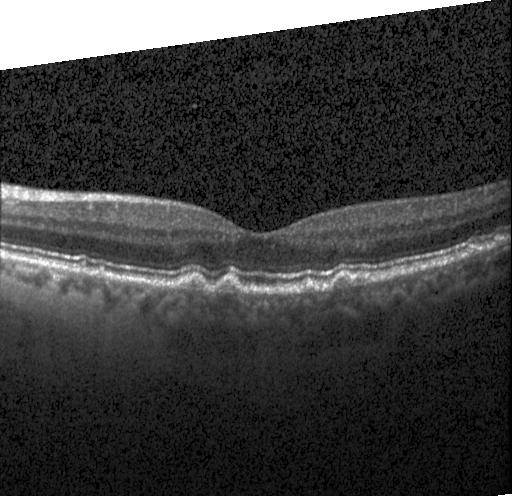 Optical coherence tomography B-scan · spectral-domain OCT · macular scan · acquired on a Heidelberg Spectralis
The scan shows multiple drusen.